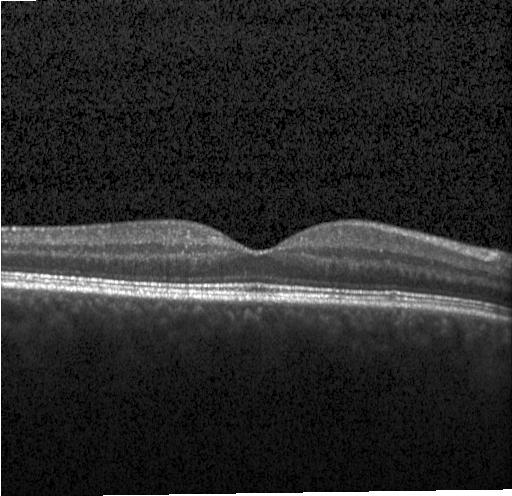
Finding: no evidence of choroidal neovascularization, diabetic macular edema, or drusen.